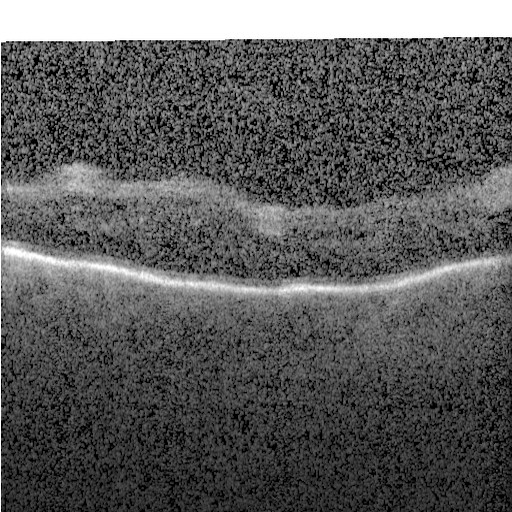 Macular OCT demonstrating DME.